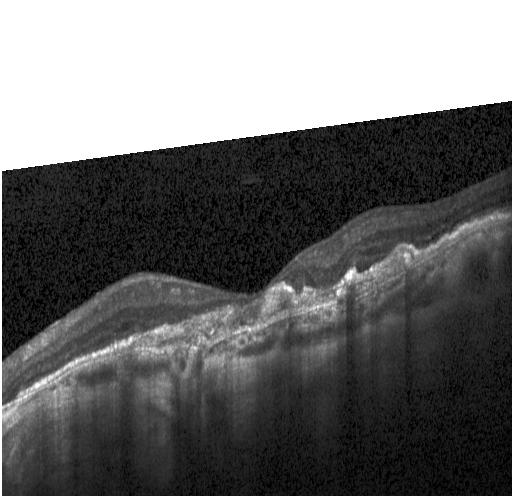

Spectral-domain optical coherence tomography · centered on the fovea · optical coherence tomography B-scan — Macular OCT: choroidal neovascularization.